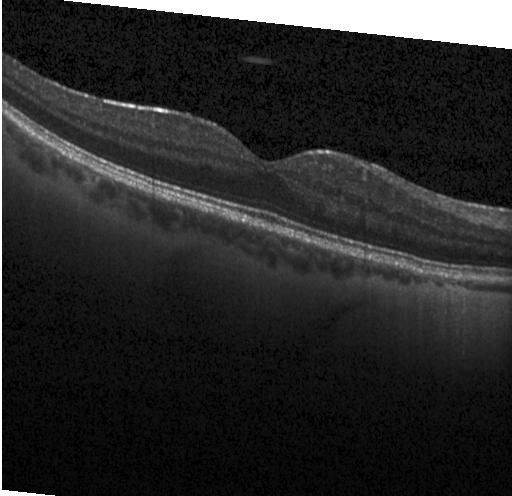

OCT scan showing no CNV, no DME, and no drusen.